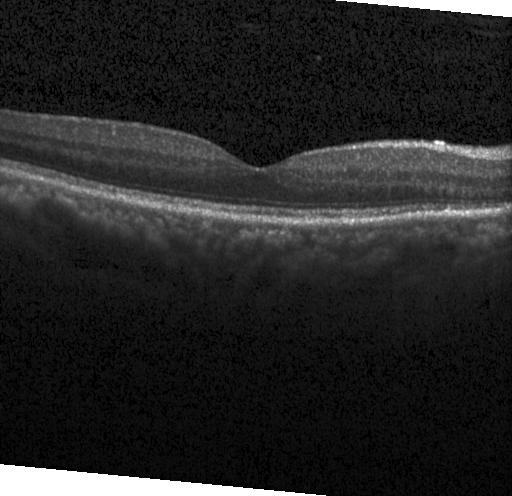 Horizontal scan through the fovea · acquired on a Heidelberg Spectralis · retinal OCT cross-section.
OCT finding: neither choroidal neovascularization, diabetic macular edema, nor drusen.